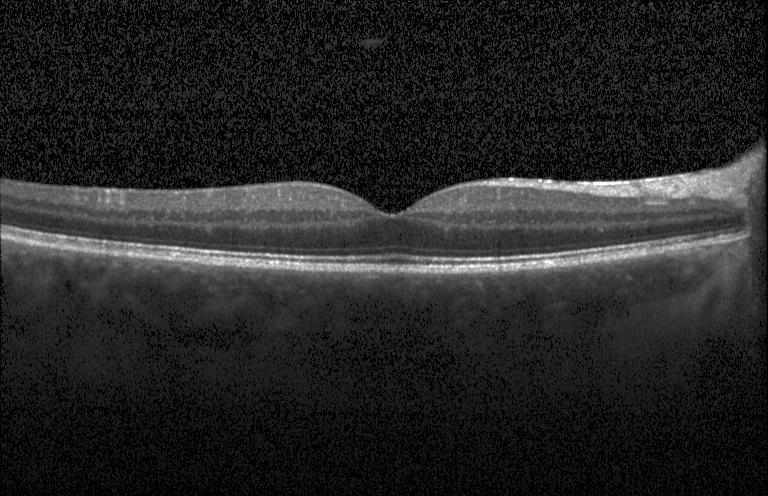 Assessment: no evidence of CNV, DME, or drusen.